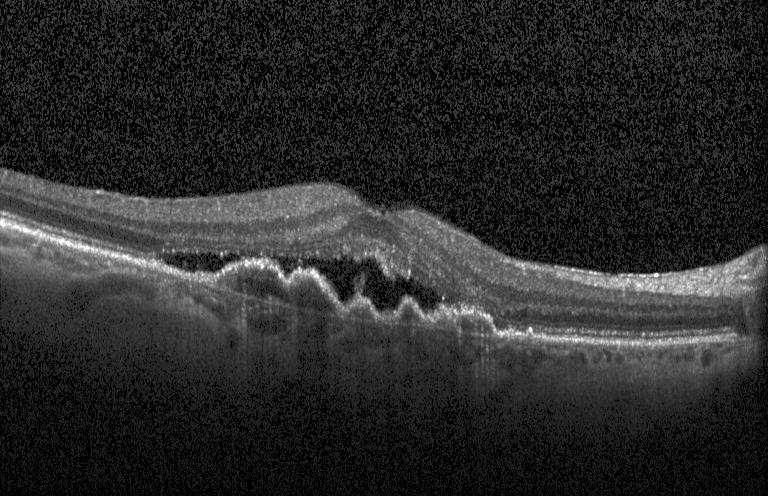 Dx: choroidal neovascularization (CNV).